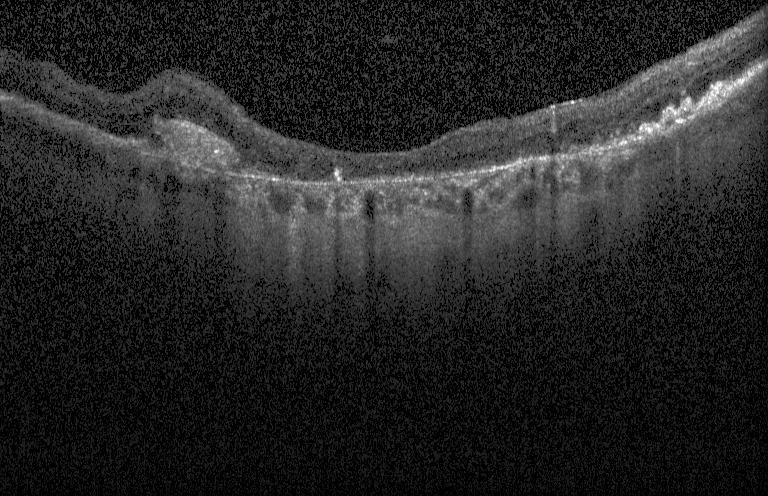

Spectral-domain optical coherence tomography; retinal OCT B-scan; horizontal scan through the fovea
Diagnosis: a choroidal neovascular membrane.